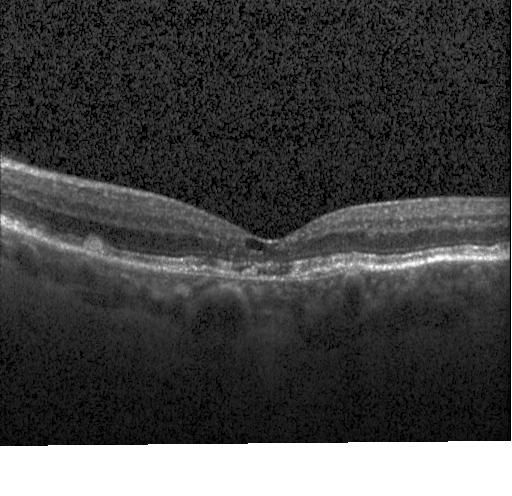
Optical coherence tomography scan, Heidelberg Spectralis OCT system, SD-OCT
Macular OCT: a choroidal neovascular membrane.